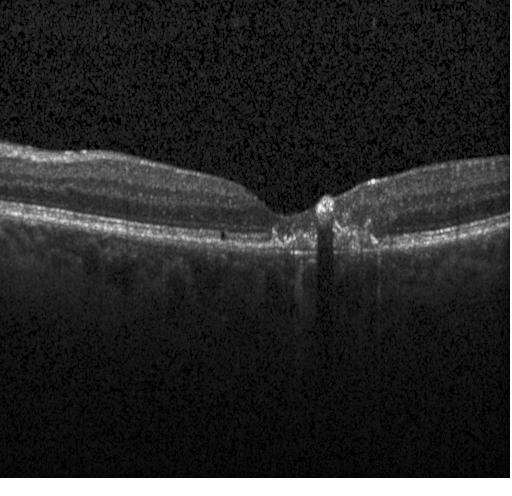 OCT scan showing CNV.